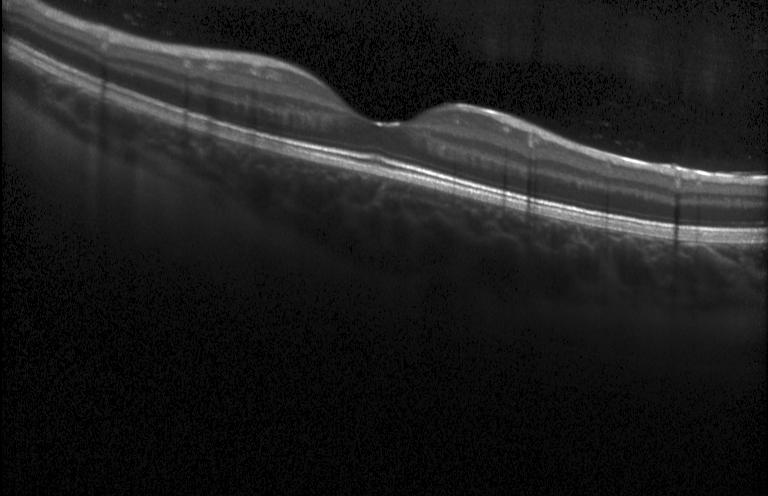 OCT finding: no CNV, no DME, and no drusen.